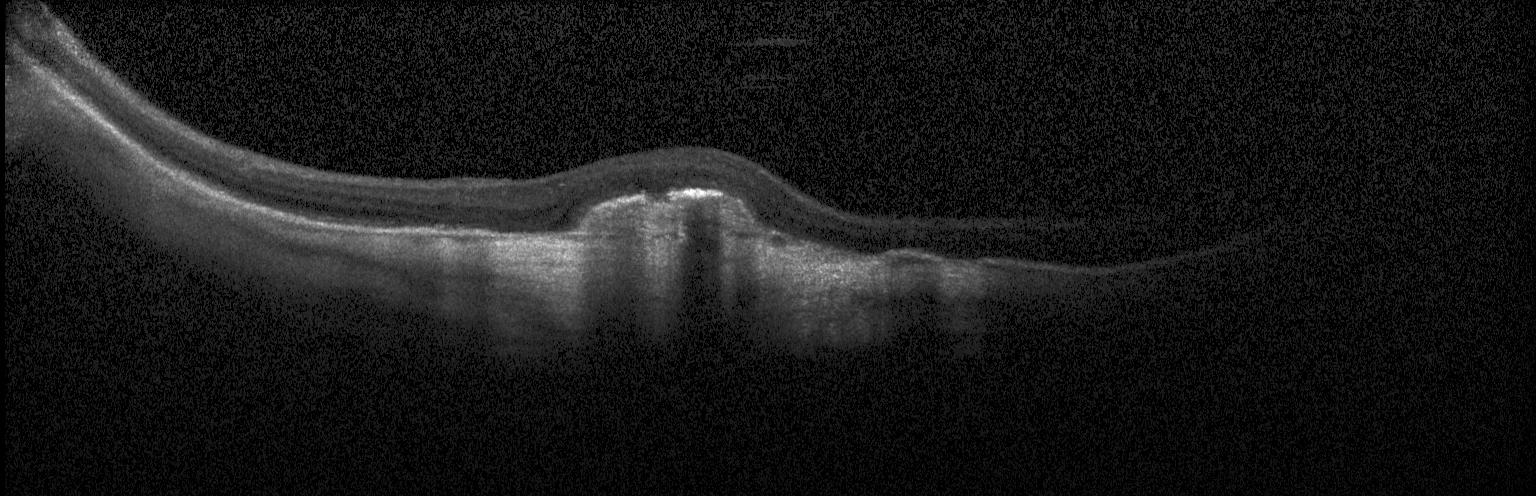 Heidelberg Spectralis · fovea-centered · retinal OCT cross-section. Assessment: CNV.